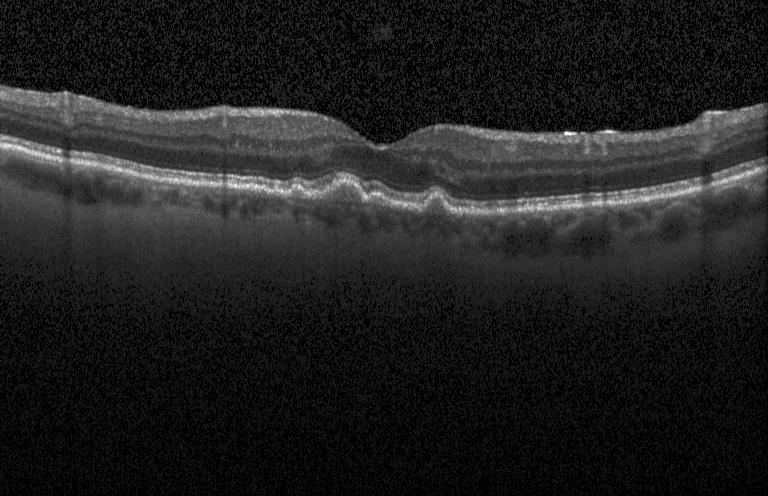 Optical coherence tomography scan. Finding: sub-RPE drusenoid deposits.